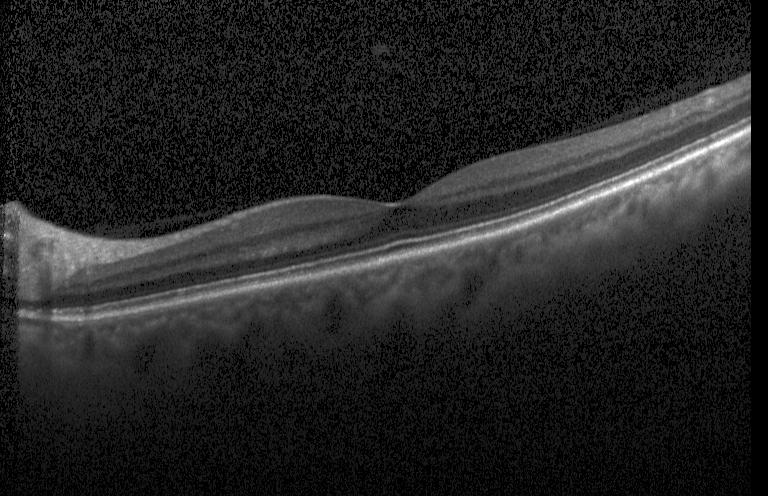
Heidelberg Spectralis; retinal OCT B-scan.
Macular OCT: neither choroidal neovascularization, diabetic macular edema, nor drusen.